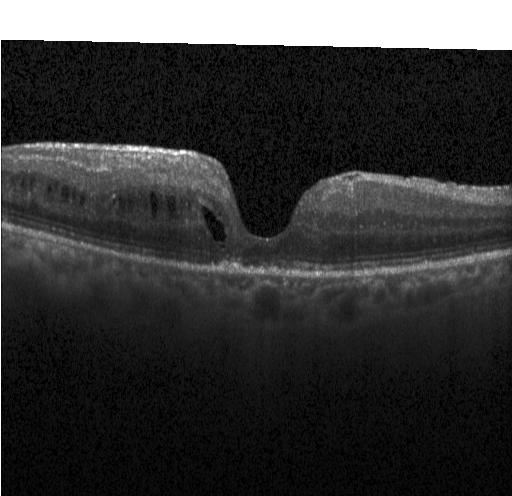 Spectral-domain OCT · OCT B-scan.
Diagnosis: diabetic macular edema.